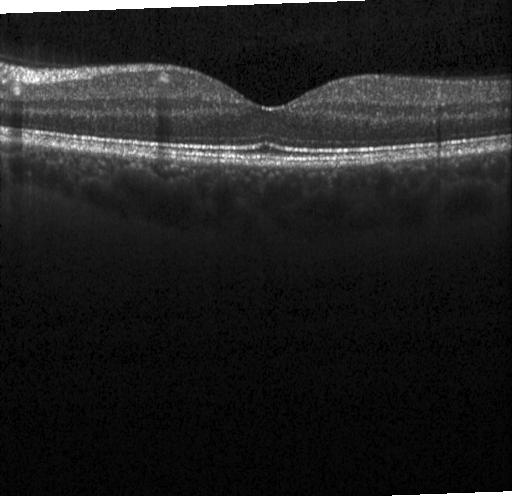

Spectral-domain OCT B-scan: no choroidal neovascularization, no diabetic macular edema, and no drusen.